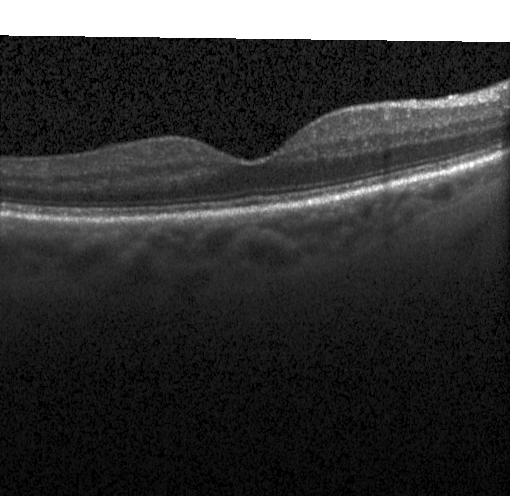

Impression: no choroidal neovascularization, diabetic macular edema, or drusen.